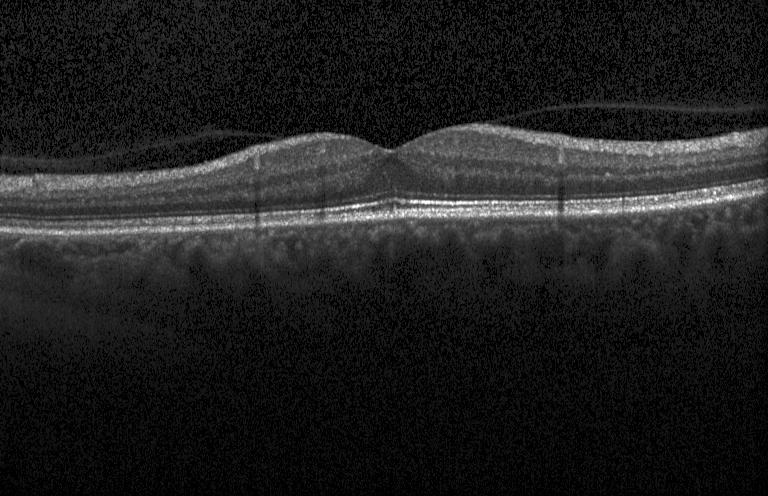
Diagnosis: no choroidal neovascularization, diabetic macular edema, or drusen.